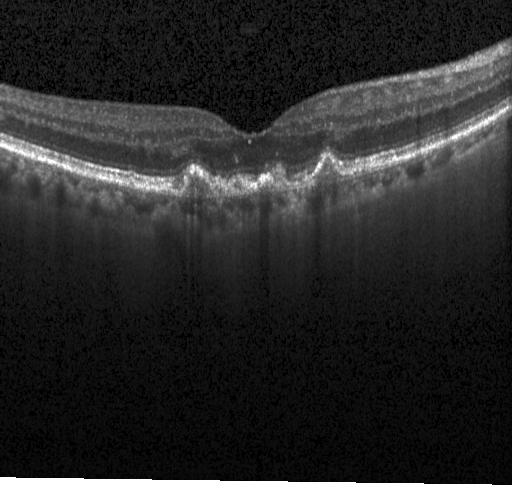
OCT B-scan, spectral-domain optical coherence tomography, Heidelberg Spectralis OCT system, horizontal scan through the fovea
Diagnosis: drusen.